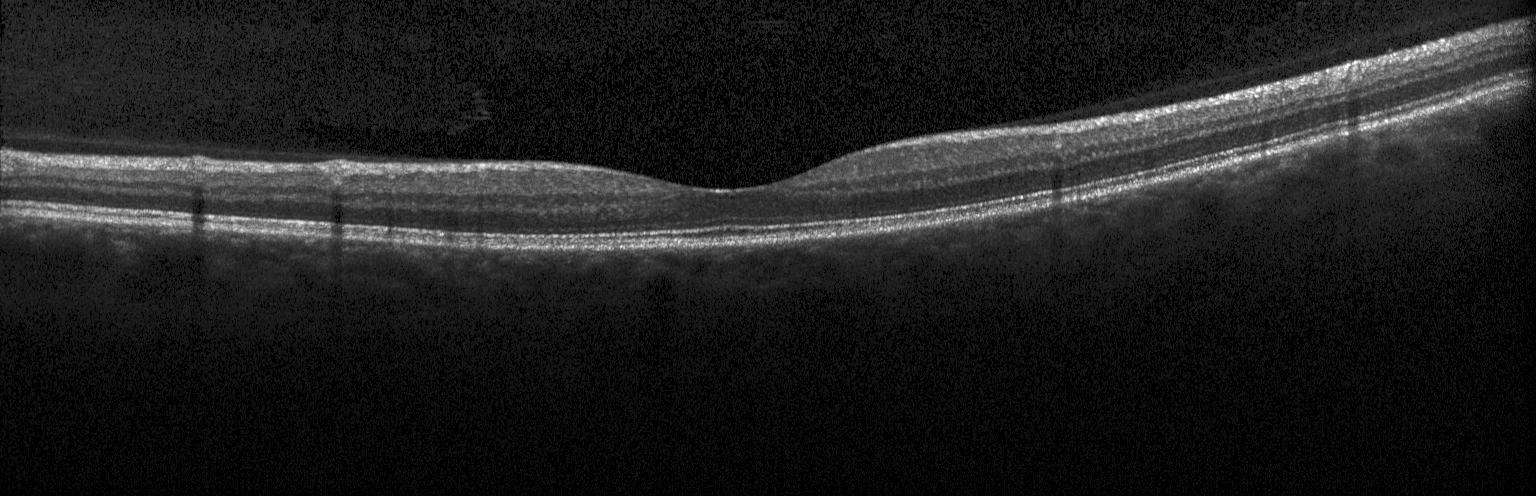 Impression: neither choroidal neovascularization, diabetic macular edema, nor drusen.